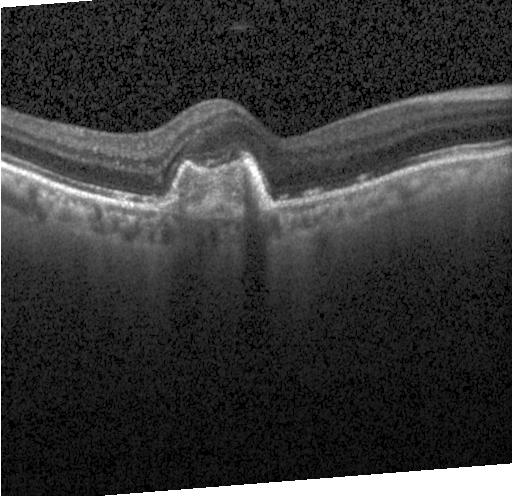
Retinal OCT cross-section showing a choroidal neovascular membrane.